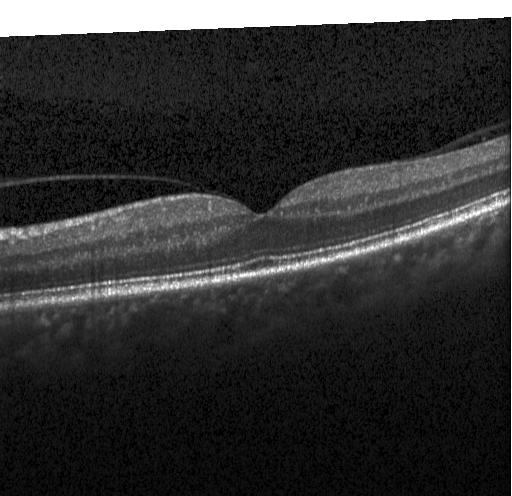

Optical coherence tomography B-scan. Finding: no evidence of CNV, DME, or drusen.